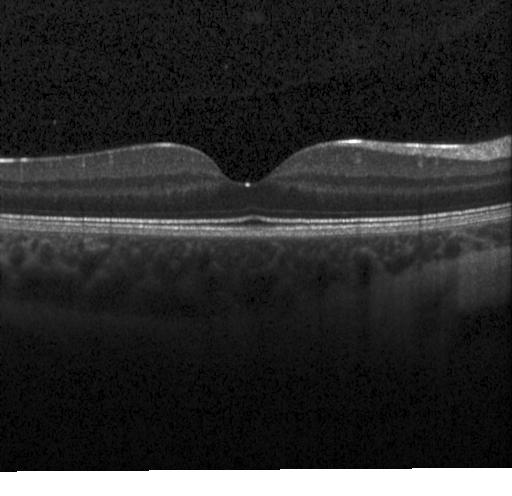
No CNV, no DME, and no drusen.